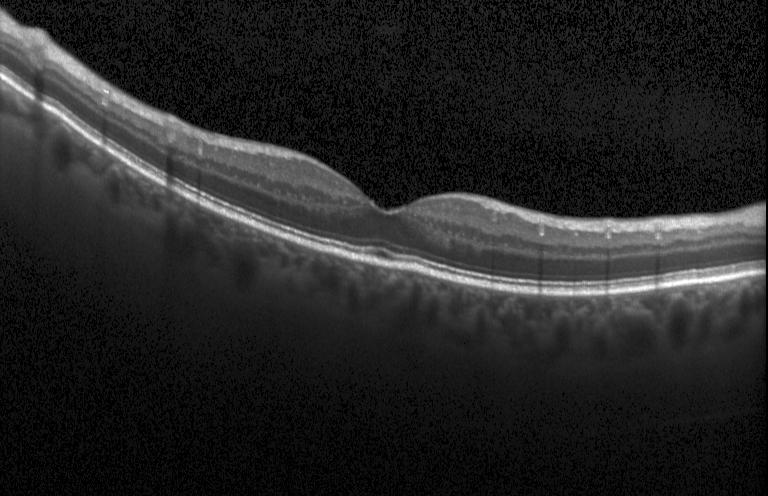 Dx: neither choroidal neovascularization, diabetic macular edema, nor drusen.